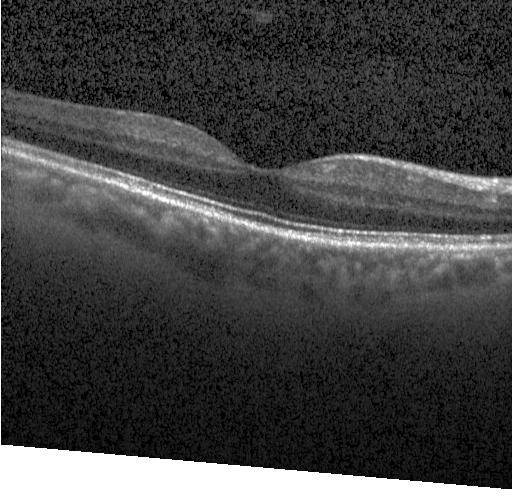
Instrument: Heidelberg Spectralis; horizontal scan through the fovea; spectral-domain optical coherence tomography; optical coherence tomography scan.
This B-scan demonstrates no evidence of choroidal neovascularization, diabetic macular edema, or drusen.